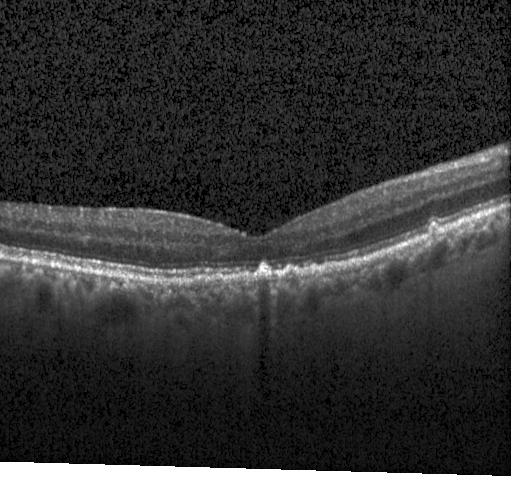

Diagnosis: sub-RPE drusenoid deposits.